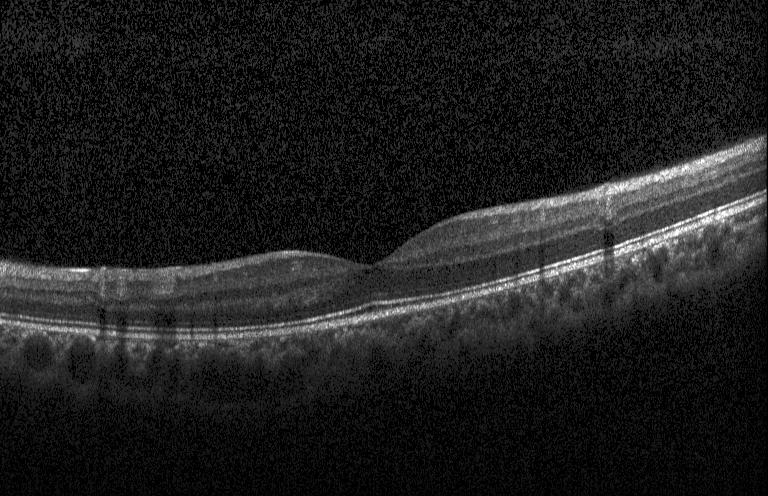

Retinal OCT cross-section, macular scan, SD-OCT
No evidence of choroidal neovascularization, diabetic macular edema, or drusen.